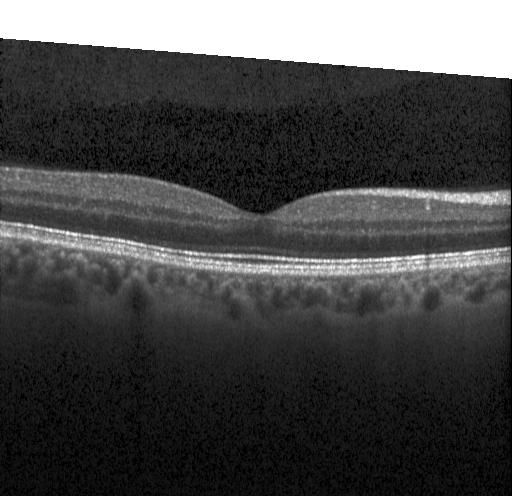

SD-OCT, fovea-centered, acquired on a Heidelberg Spectralis, OCT B-scan. No evidence of choroidal neovascularization, diabetic macular edema, or drusen.